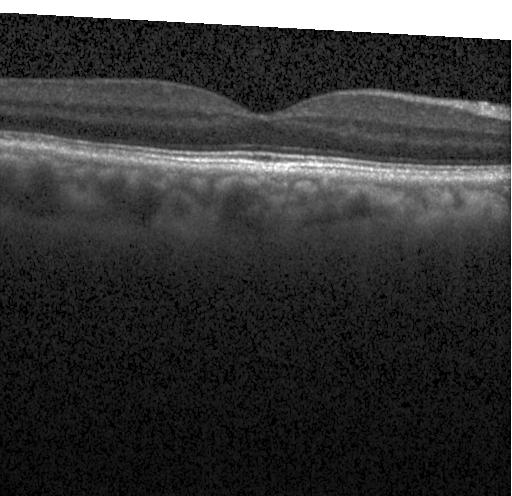
Retinal OCT cross-section showing neither choroidal neovascularization, diabetic macular edema, nor drusen.